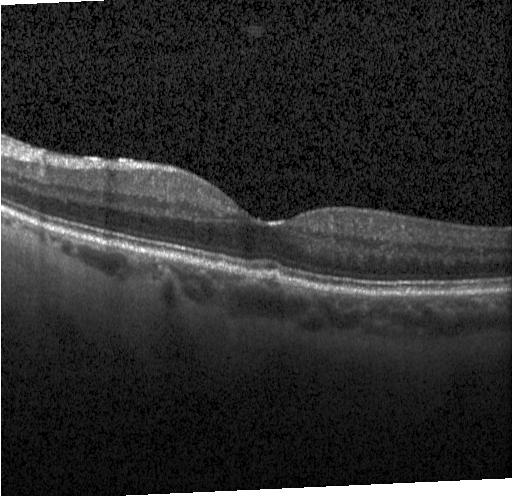 OCT B-scan. OCT finding: no choroidal neovascularization, no diabetic macular edema, and no drusen.